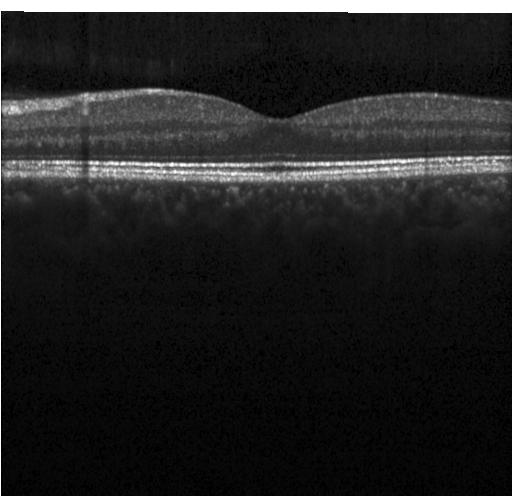

SD-OCT, OCT line scan — Impression: no evidence of CNV, DME, or drusen.